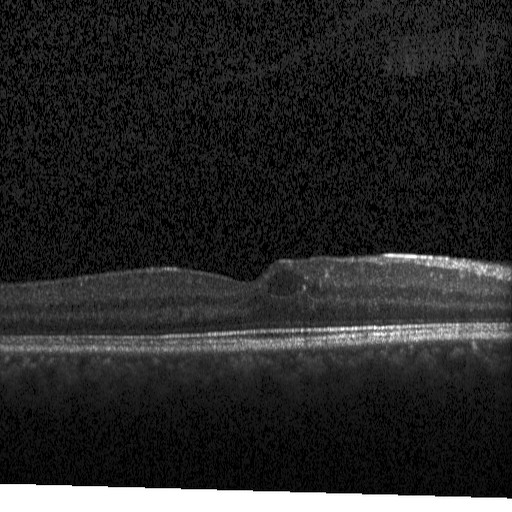

Horizontal scan through the fovea. Heidelberg Spectralis. Spectral-domain OCT. Optical coherence tomography scan. Dx: DME.